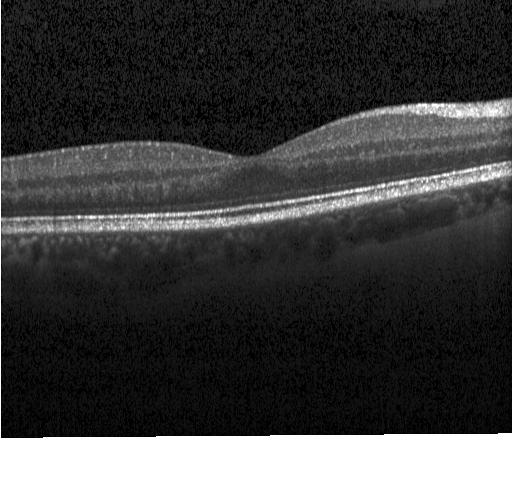
Acquired on a Heidelberg Spectralis. Retinal OCT B-scan. Spectral-domain optical coherence tomography. Fovea-centered
Impression: neither choroidal neovascularization, diabetic macular edema, nor drusen.